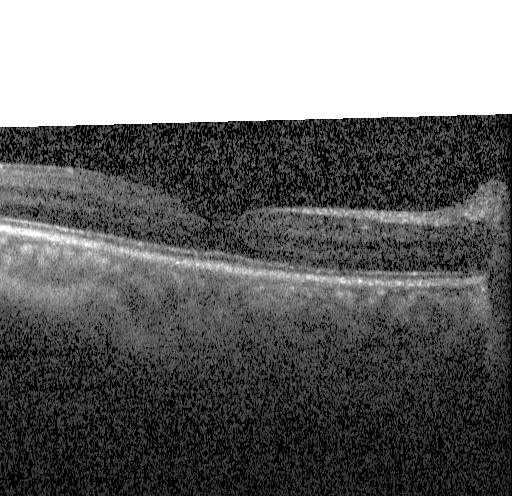

Macular OCT demonstrating no evidence of CNV, DME, or drusen.